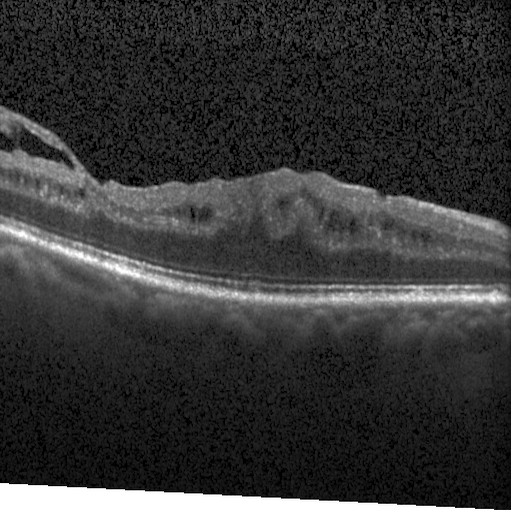
OCT finding: diabetic macular edema.